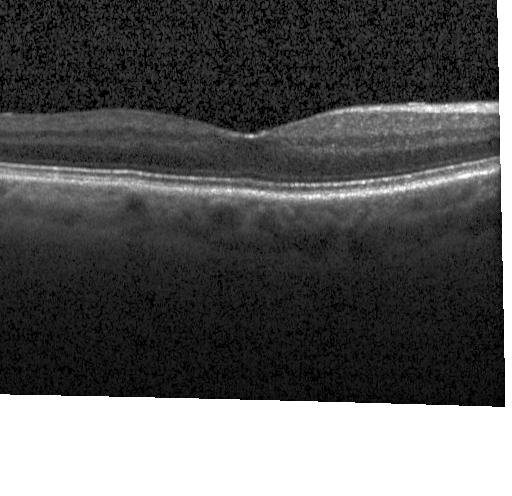 Retinal OCT B-scan · Heidelberg Spectralis — Finding: no evidence of choroidal neovascularization, diabetic macular edema, or drusen.